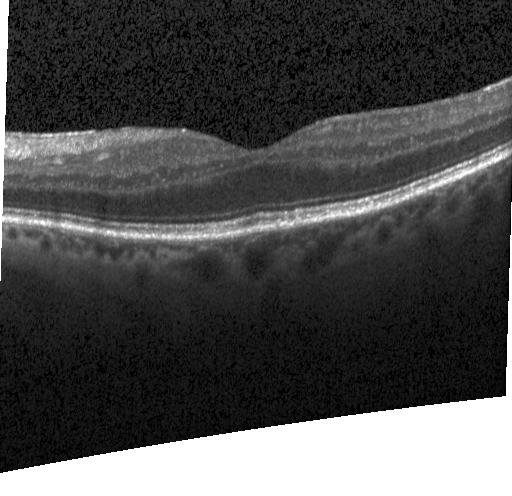
Impression: no choroidal neovascularization, diabetic macular edema, or drusen.